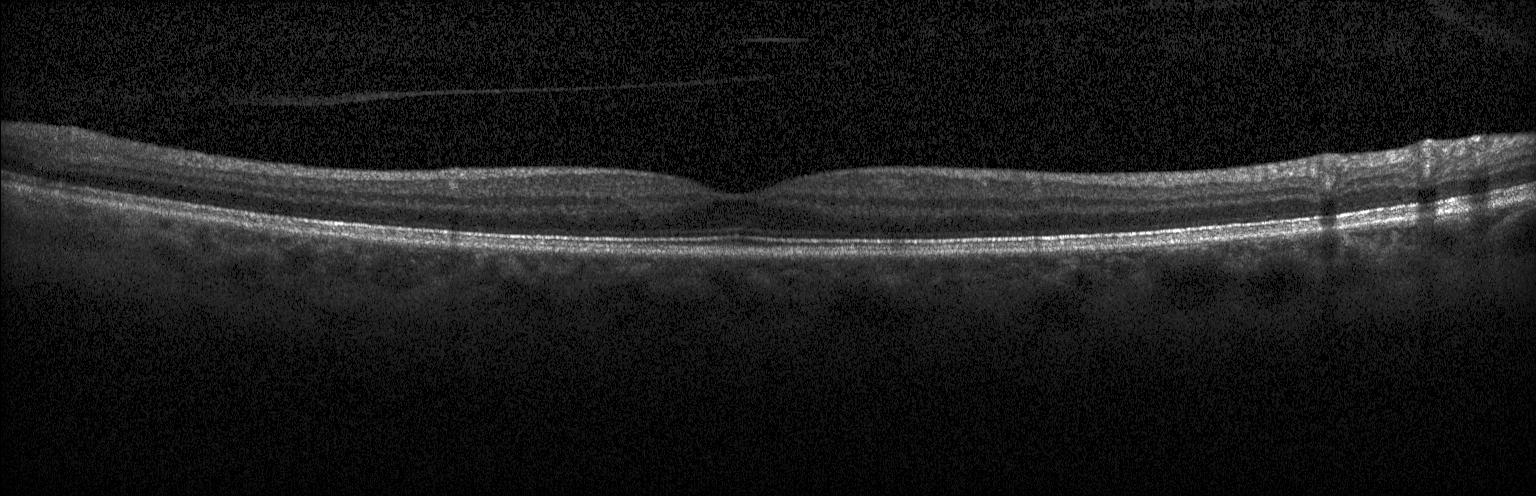
Finding: neither CNV, DME, nor drusen.